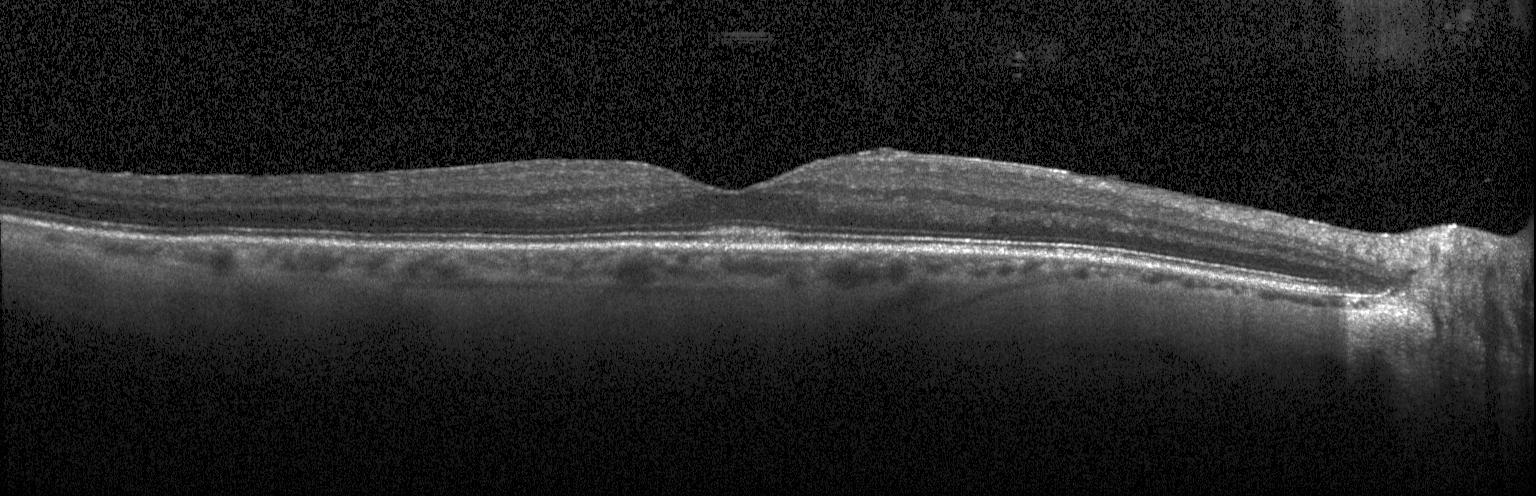 Impression: no evidence of choroidal neovascularization, diabetic macular edema, or drusen.